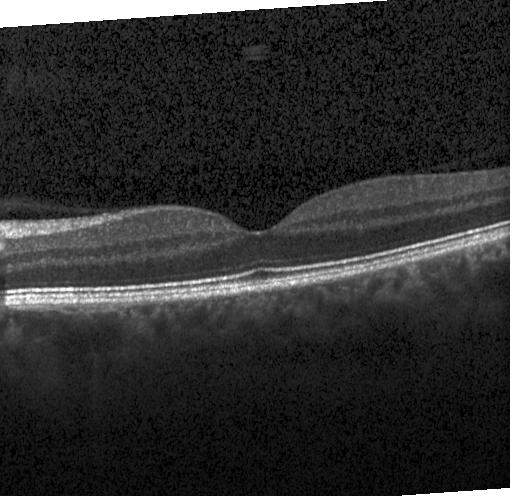 Macular OCT: no CNV, no DME, and no drusen.